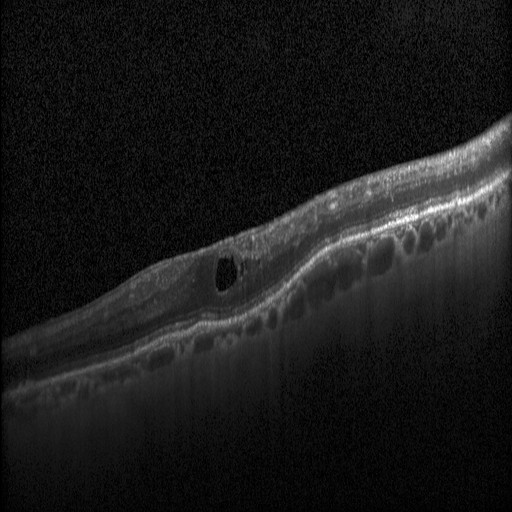
Fovea-centered, Heidelberg Spectralis, OCT B-scan
Assessment: diabetic macular edema (DME).